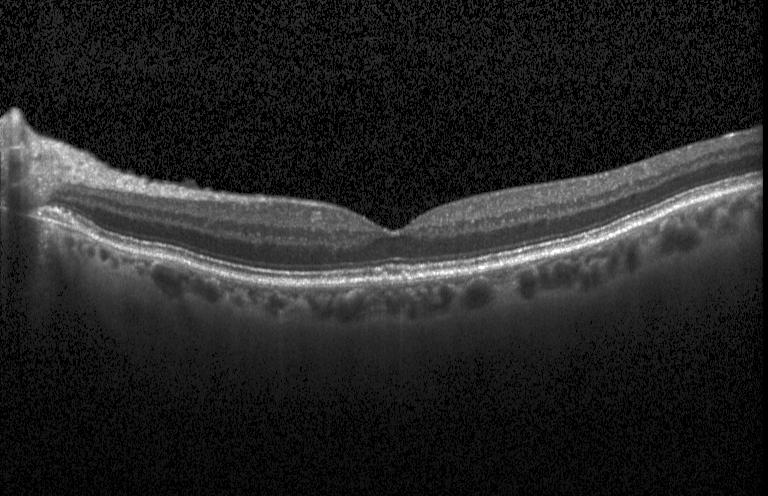
Finding: no evidence of choroidal neovascularization, diabetic macular edema, or drusen.